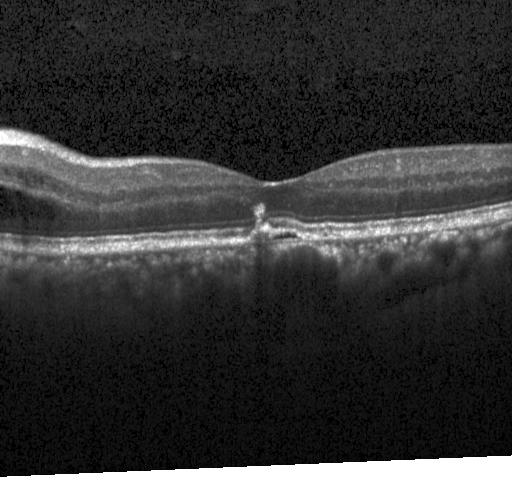 Spectral-domain optical coherence tomography, OCT B-scan, through the macula, Heidelberg Spectralis — The scan shows choroidal neovascularization.